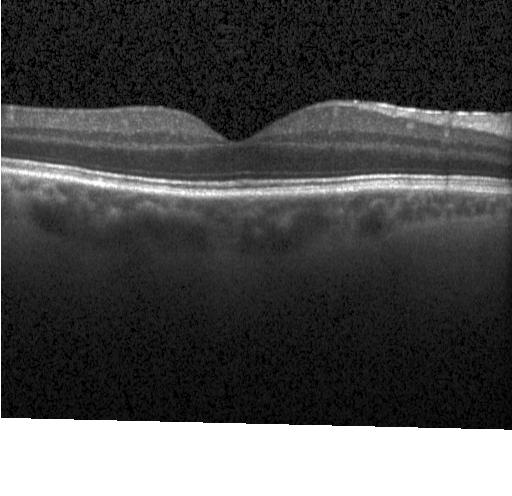 Macular scan, OCT B-scan, SD-OCT.
Impression: no CNV, no DME, and no drusen.